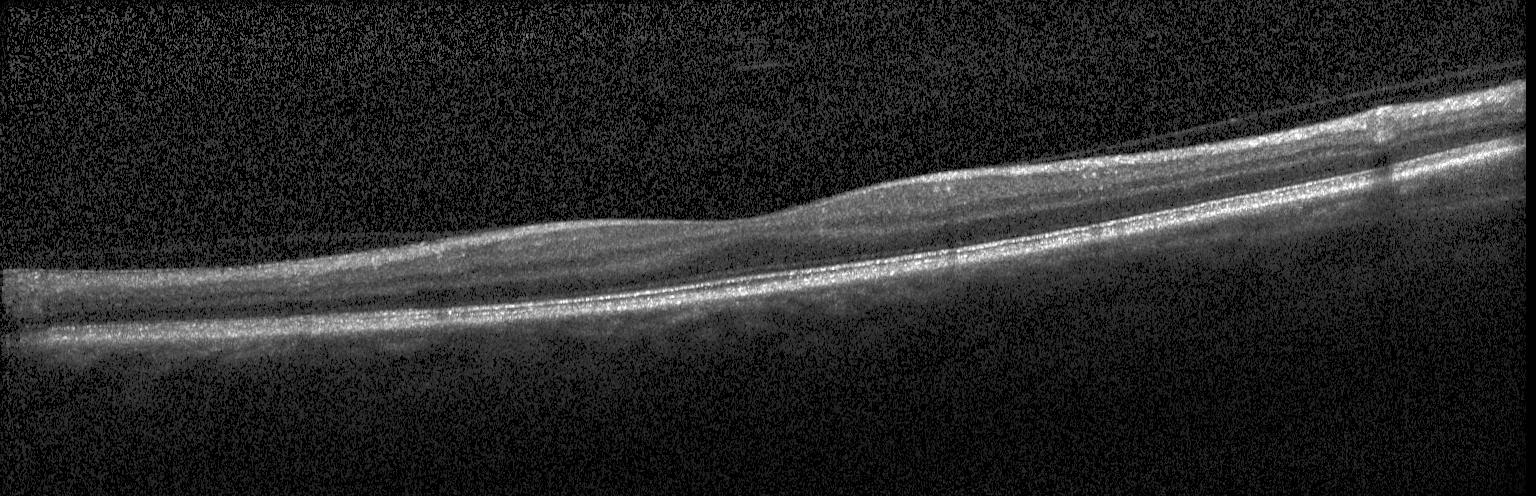 Retinal OCT cross-section; acquired on a Heidelberg Spectralis
Finding: no choroidal neovascularization, diabetic macular edema, or drusen.